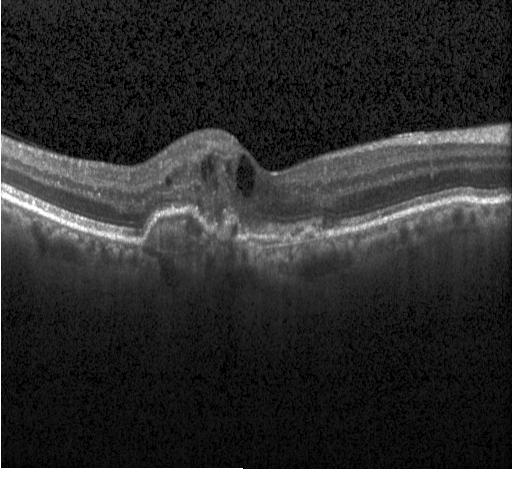 Horizontal scan through the fovea. OCT line scan — OCT finding: a choroidal neovascular membrane.